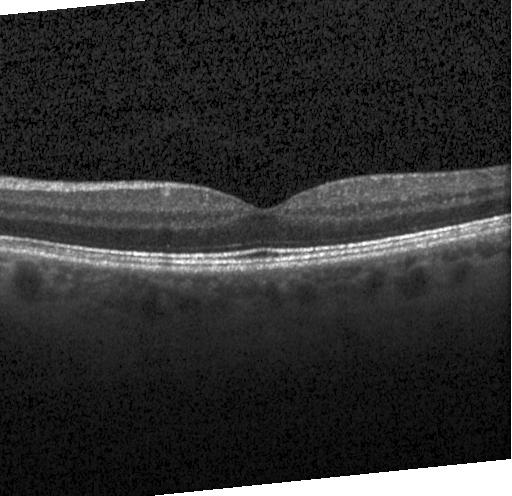
OCT B-scan; horizontal scan through the fovea. OCT finding: no choroidal neovascularization, diabetic macular edema, or drusen.